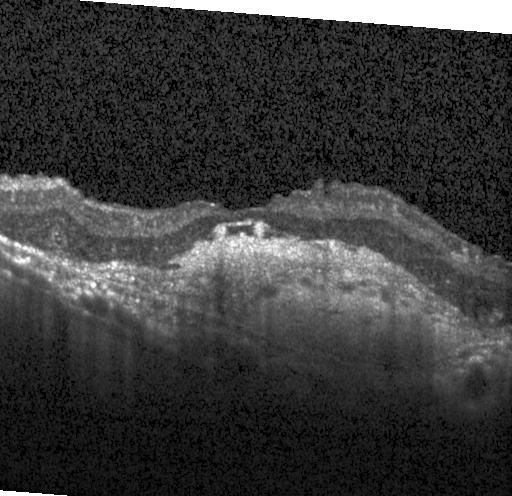

The scan shows choroidal neovascularization (CNV).